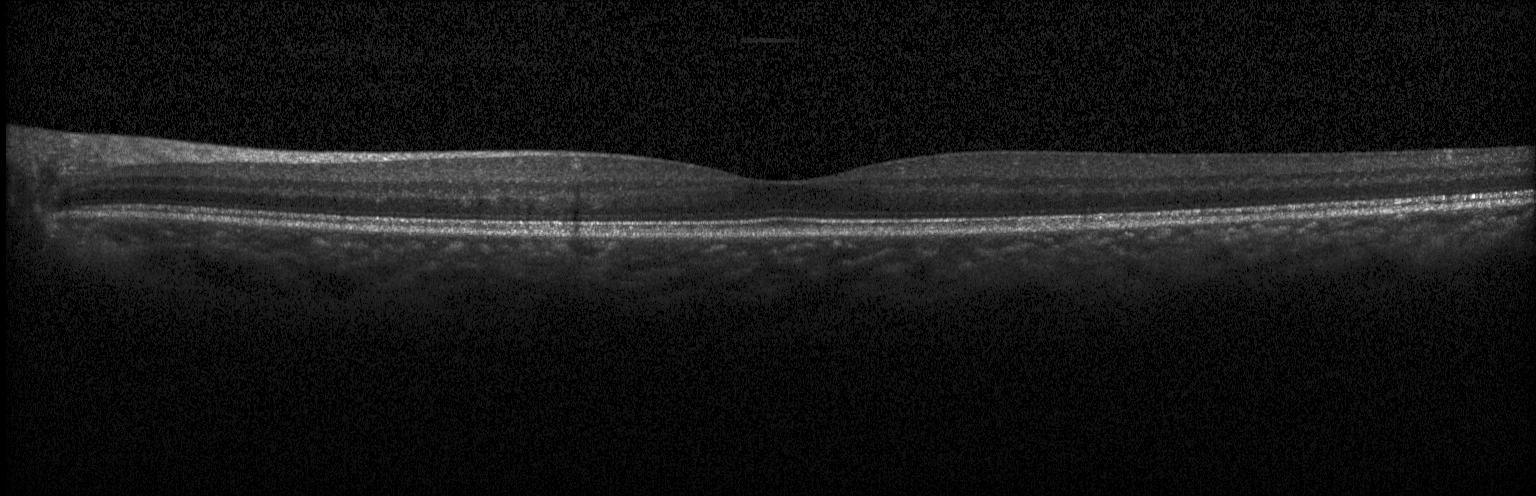 Retinal OCT B-scan · SD-OCT
Impression: no choroidal neovascularization, no diabetic macular edema, and no drusen.